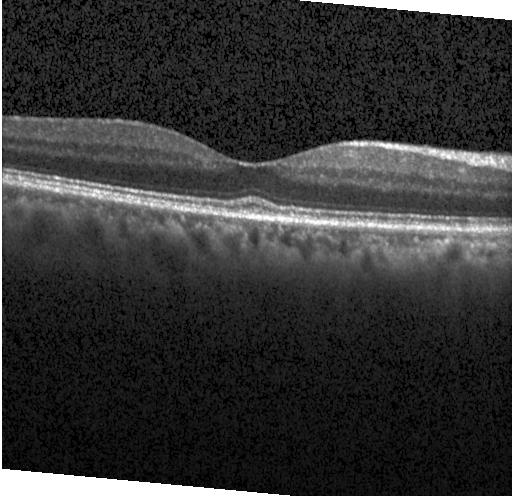
Retinal OCT cross-section showing neither CNV, DME, nor drusen.